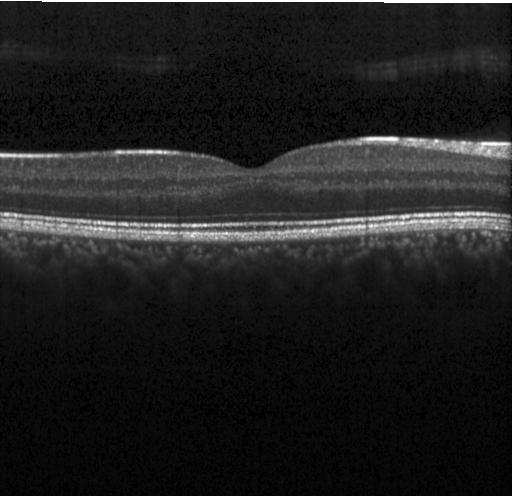
Macular scan; optical coherence tomography B-scan; instrument: Heidelberg Spectralis
This B-scan demonstrates no evidence of choroidal neovascularization, diabetic macular edema, or drusen.